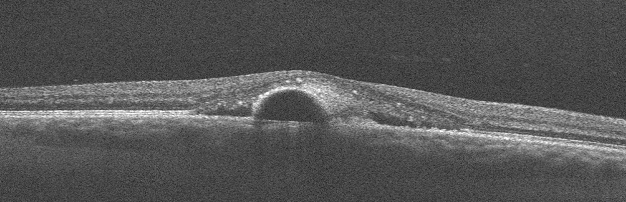 Dx: age-related macular degeneration (AMD).